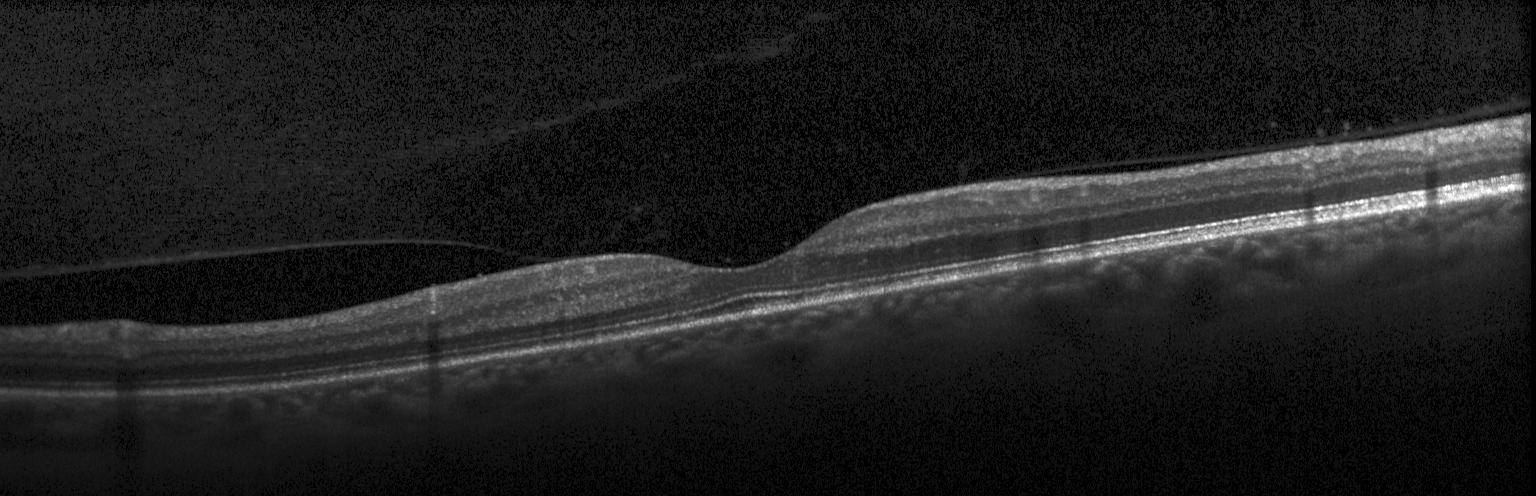 Retinal OCT cross-section; centered on the fovea; acquired on a Heidelberg Spectralis. Finding: no choroidal neovascularization, no diabetic macular edema, and no drusen.